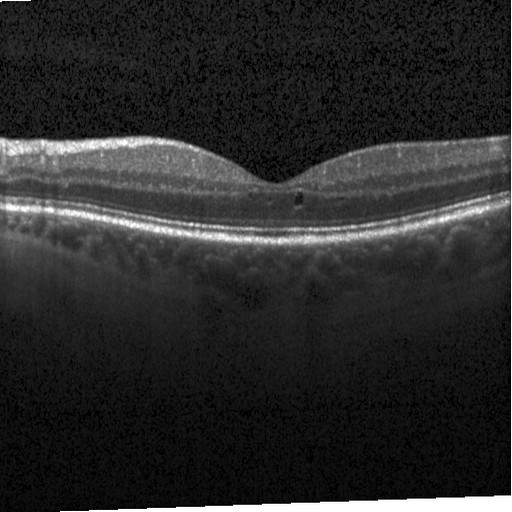

OCT line scan — Finding: diabetic macular edema.